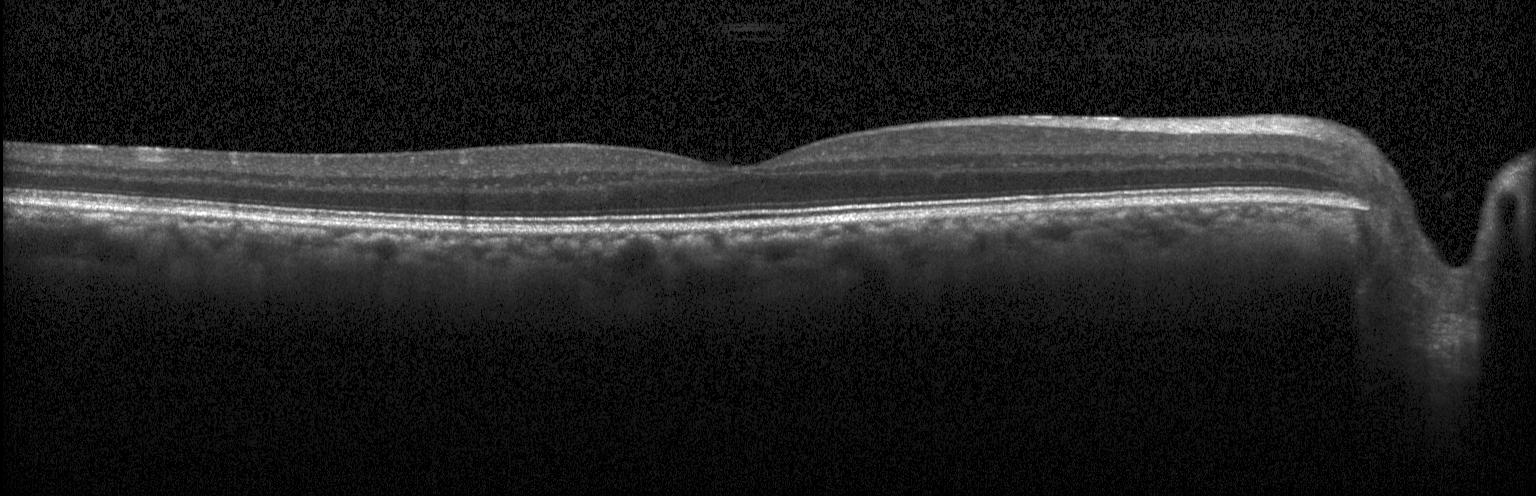
Spectral-domain optical coherence tomography; retinal OCT B-scan
OCT finding: no evidence of choroidal neovascularization, diabetic macular edema, or drusen.